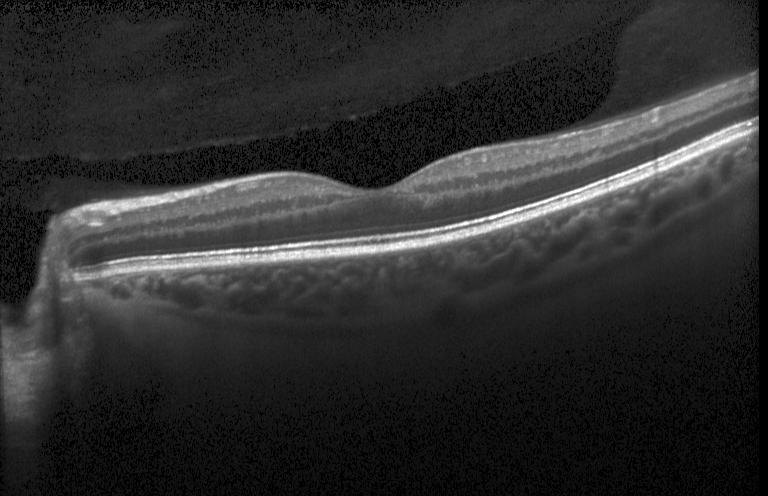 OCT scan showing no evidence of CNV, DME, or drusen.